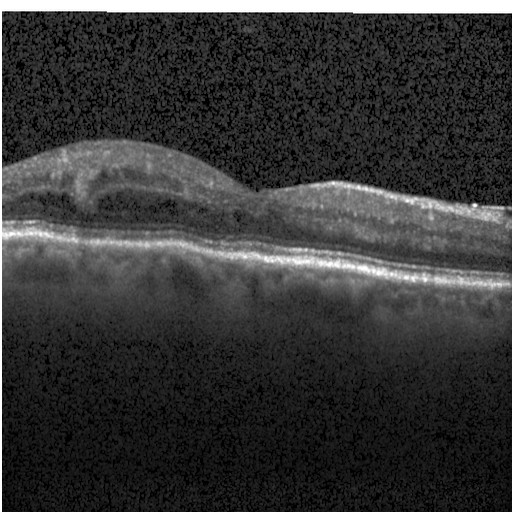 Retinal OCT B-scan
The scan shows diabetic macular edema.